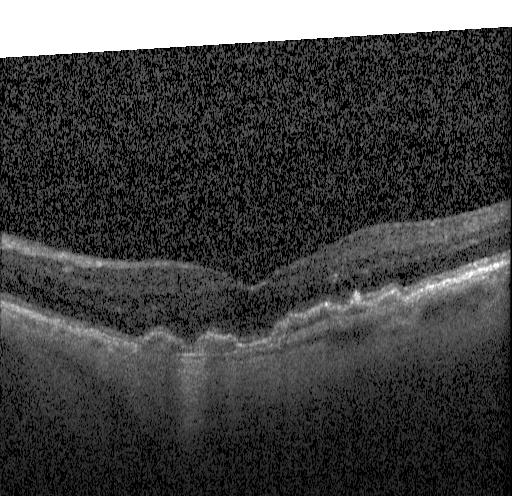
The scan shows choroidal neovascularization.